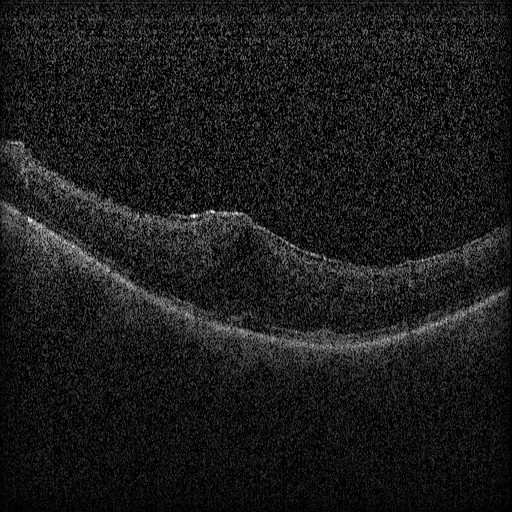

Optical coherence tomography B-scan, horizontal scan through the fovea — This B-scan demonstrates diabetic macular edema.